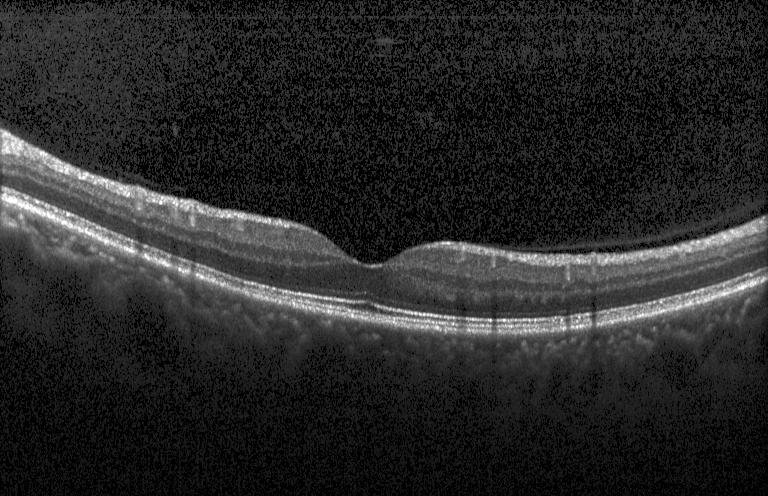 Spectral-domain optical coherence tomography · retinal OCT cross-section — Assessment: no choroidal neovascularization, diabetic macular edema, or drusen.